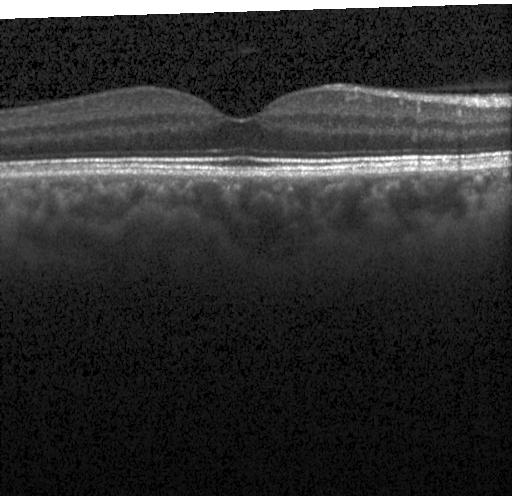
Heidelberg Spectralis OCT system. Spectral-domain optical coherence tomography. Through the macula. Optical coherence tomography B-scan. Diagnosis: no evidence of choroidal neovascularization, diabetic macular edema, or drusen.